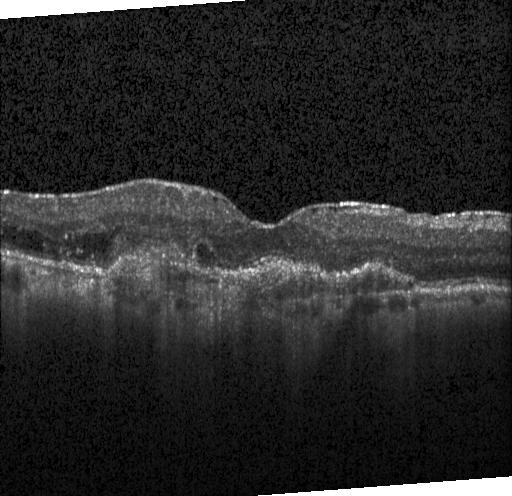

Acquired on a Heidelberg Spectralis; retinal OCT B-scan. Finding: choroidal neovascularization.